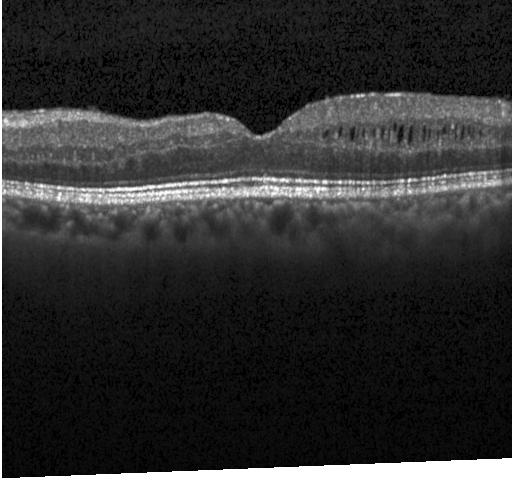 OCT B-scan. The scan shows diabetic macular edema (DME).